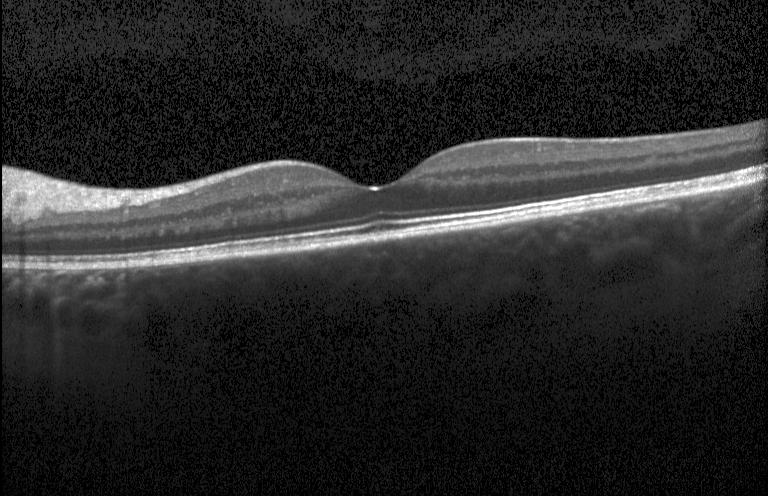
Assessment: no evidence of CNV, DME, or drusen.